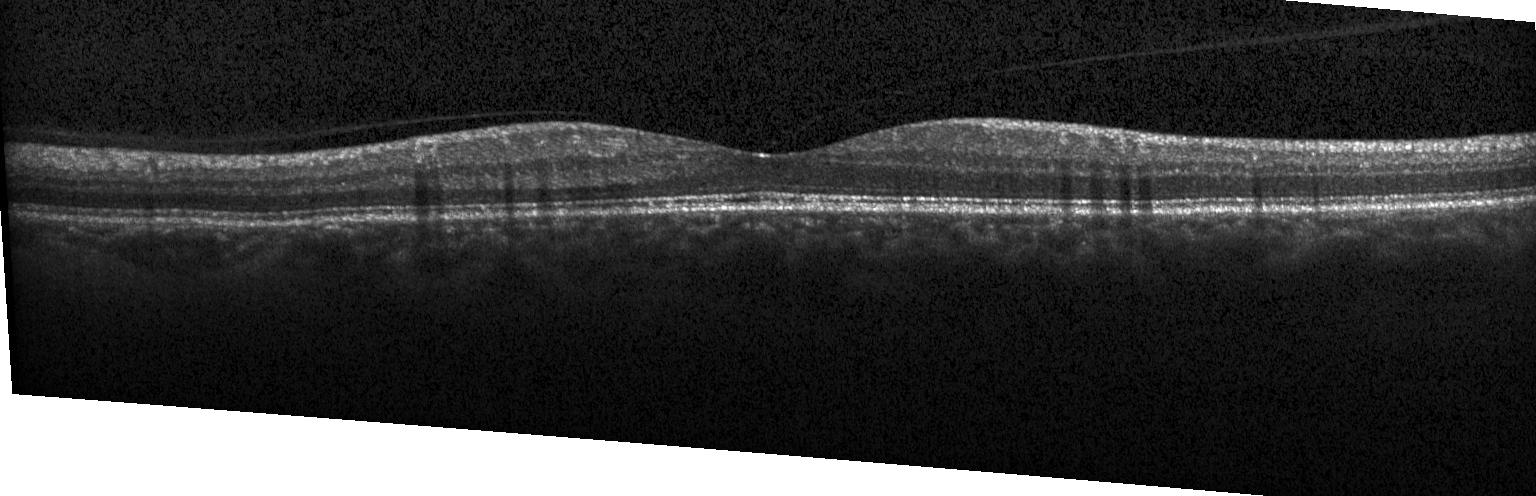

Retinal OCT cross-section
Impression: no choroidal neovascularization, no diabetic macular edema, and no drusen.